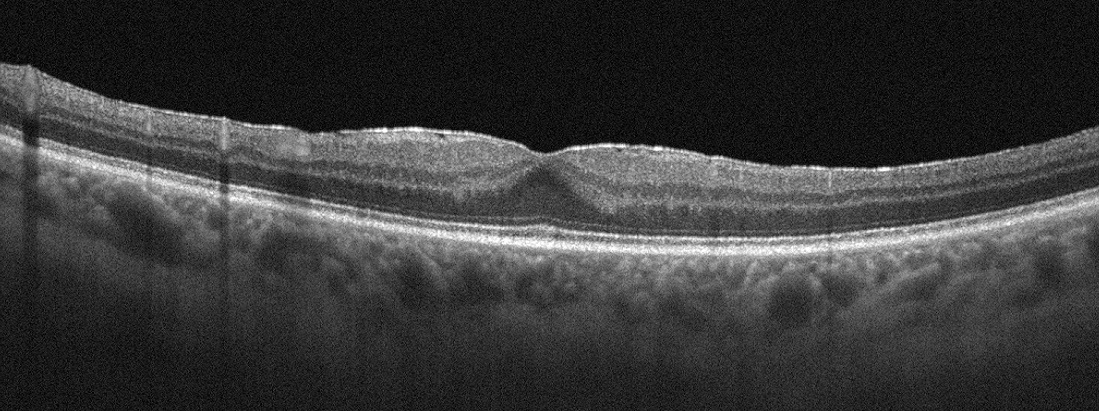
Through the macula. Optovue Avanti RTVue XR. Retinal OCT B-scan. OCT finding: epiretinal membrane.